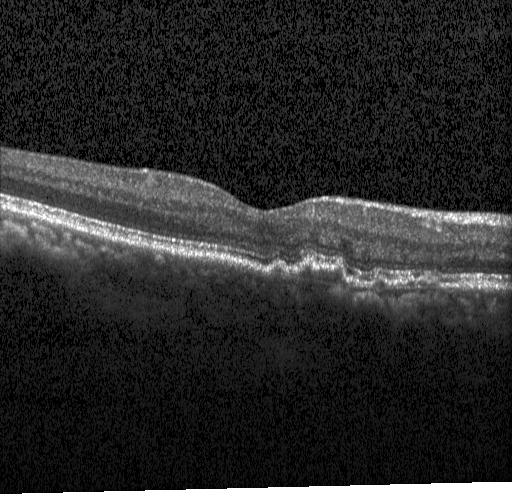
Instrument: Heidelberg Spectralis · spectral-domain optical coherence tomography · retinal OCT B-scan. Assessment: sub-RPE drusenoid deposits.